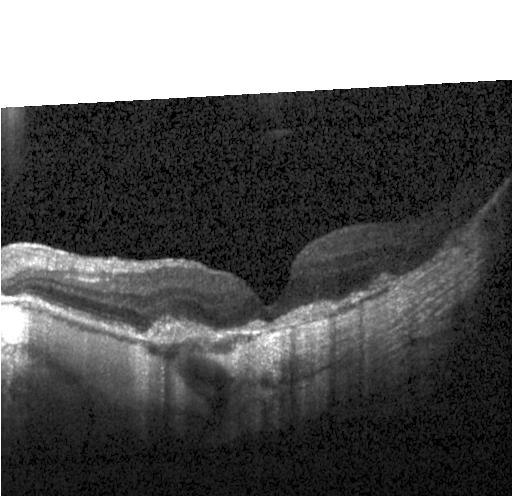 Retinal OCT B-scan · horizontal scan through the fovea — Assessment: a choroidal neovascular membrane.